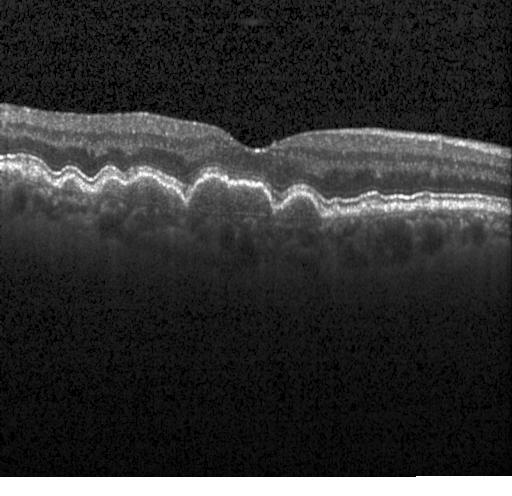 Impression: sub-RPE drusenoid deposits.